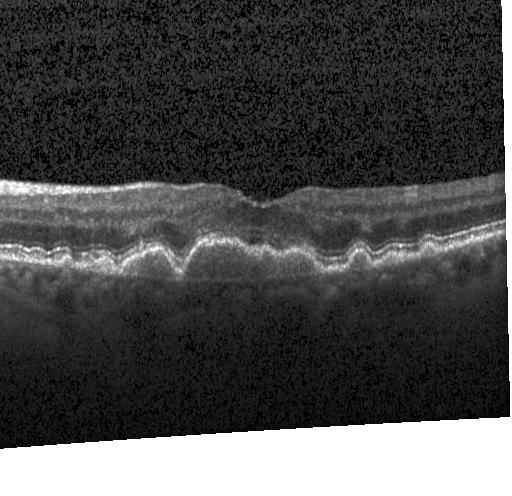
Retinal OCT cross-section. Instrument: Heidelberg Spectralis. Impression: a choroidal neovascular membrane.